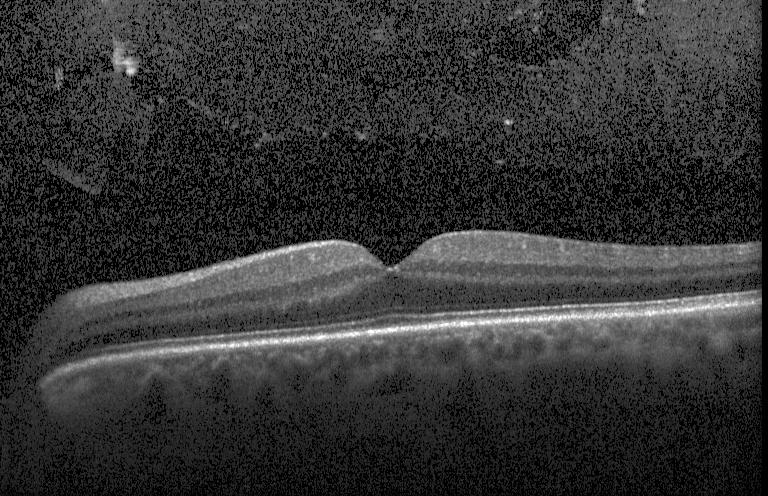 Neither choroidal neovascularization, diabetic macular edema, nor drusen.